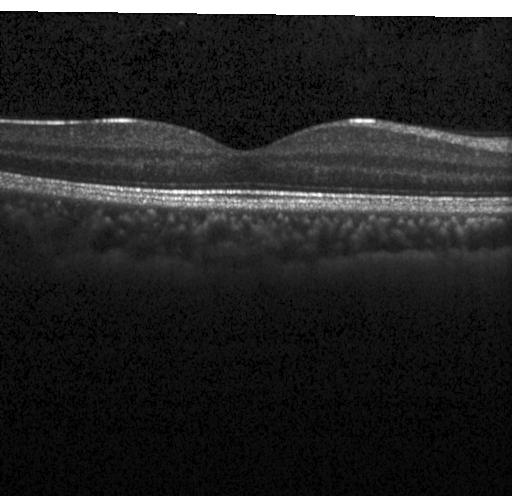
SD-OCT · optical coherence tomography B-scan · centered on the fovea
Finding: no choroidal neovascularization, diabetic macular edema, or drusen.